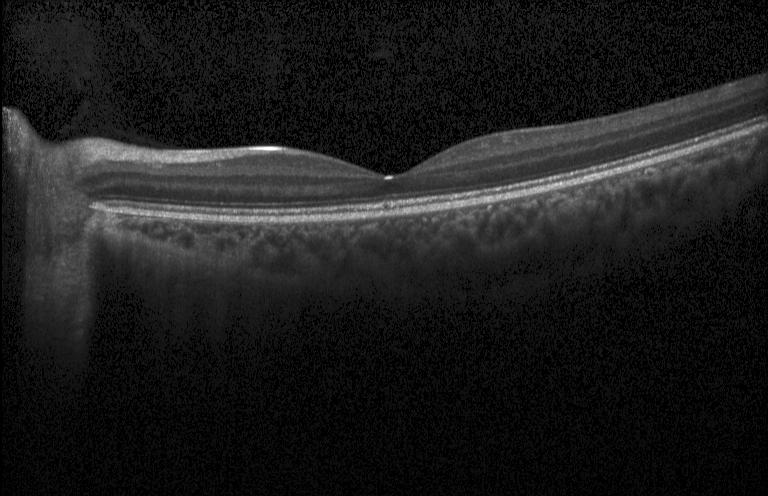

The scan shows no CNV, DME, or drusen.